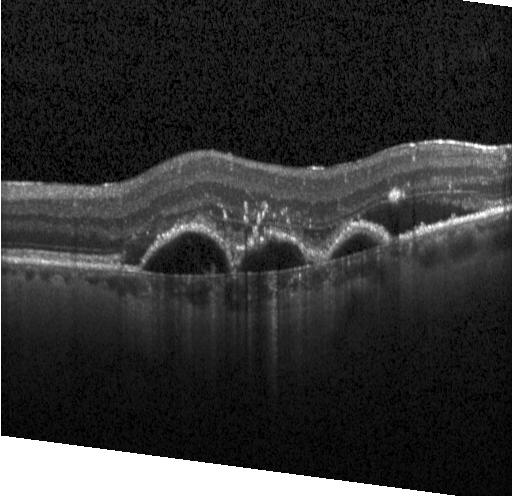
Heidelberg Spectralis OCT system. Horizontal scan through the fovea. OCT B-scan. Spectral-domain OCT — Dx: a choroidal neovascular membrane.